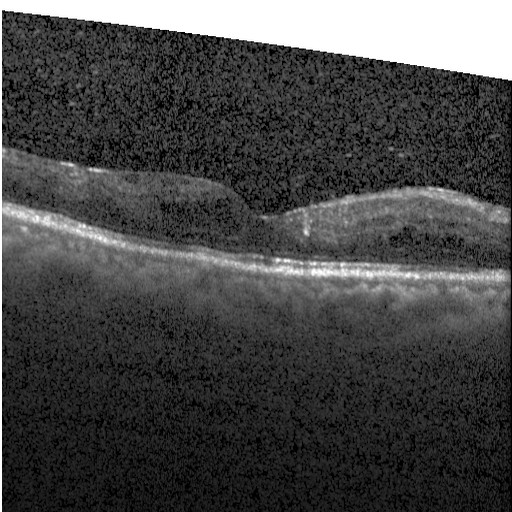
Impression: DME.